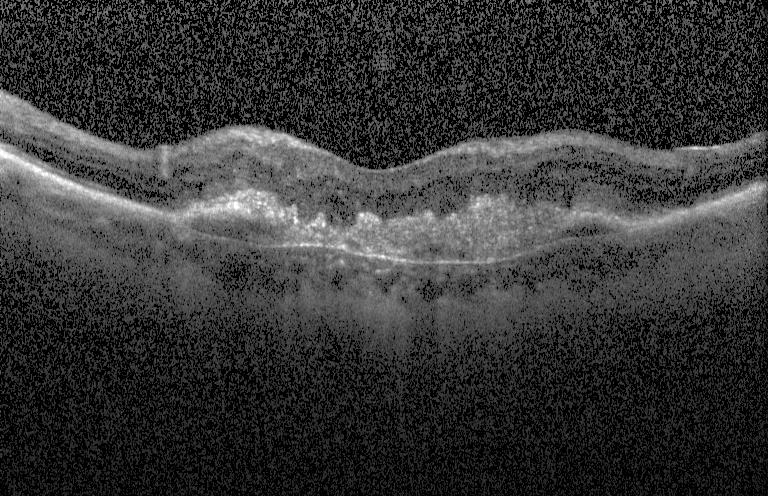 Macular OCT: a choroidal neovascular membrane.